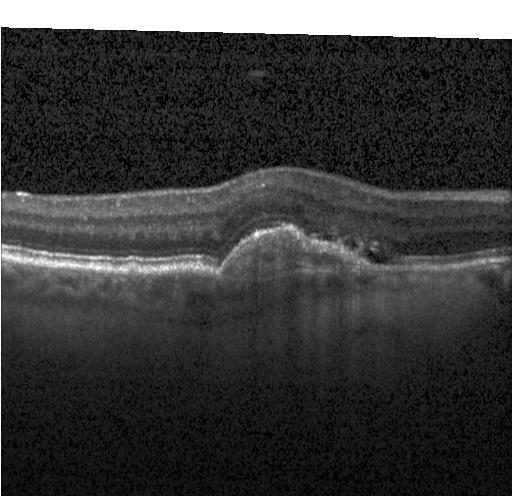

OCT line scan — Diagnosis: a choroidal neovascular membrane.